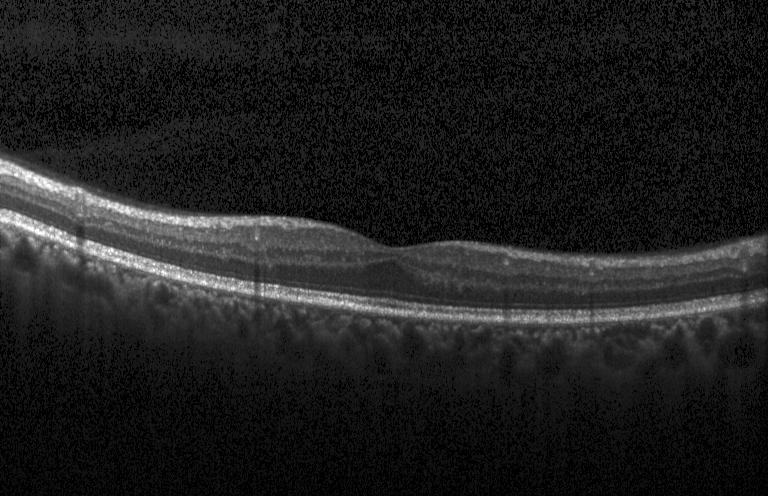 Retinal OCT cross-section showing no choroidal neovascularization, diabetic macular edema, or drusen.